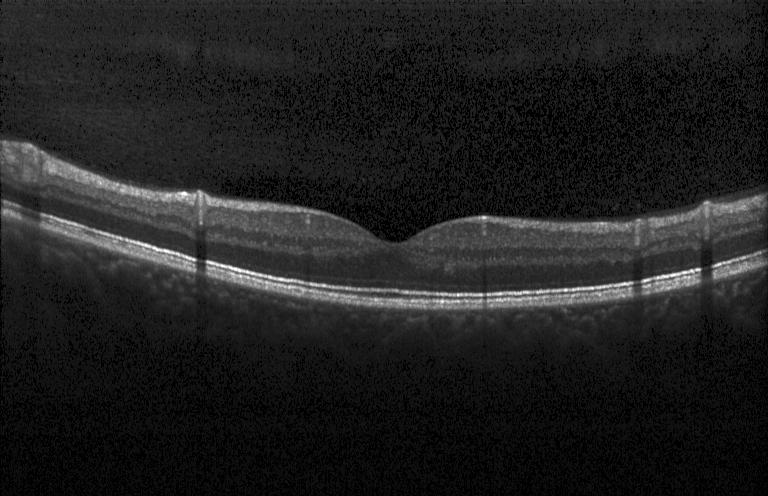

Heidelberg Spectralis OCT system. Retinal OCT B-scan. Macular scan. SD-OCT. Impression: no choroidal neovascularization, no diabetic macular edema, and no drusen.